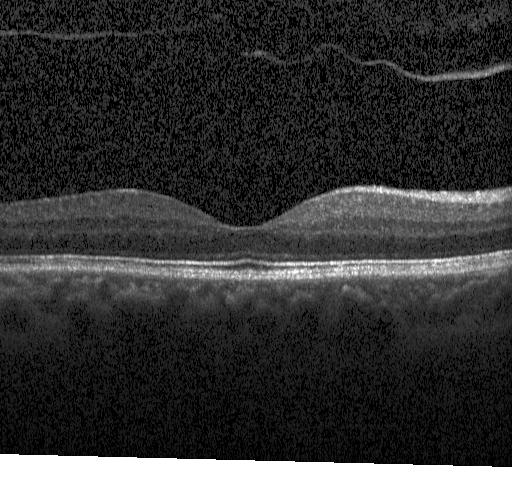

Retinal OCT cross-section showing neither choroidal neovascularization, diabetic macular edema, nor drusen.